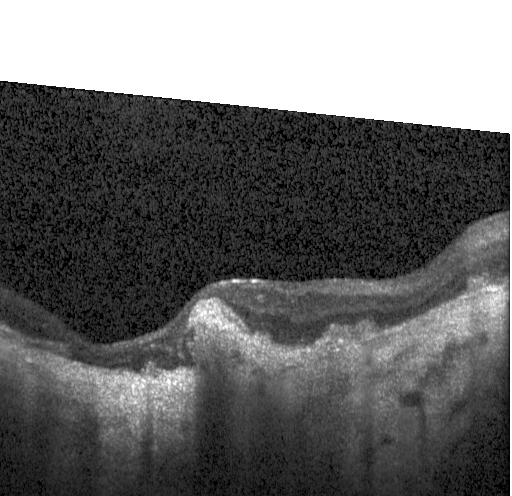

Assessment: CNV.